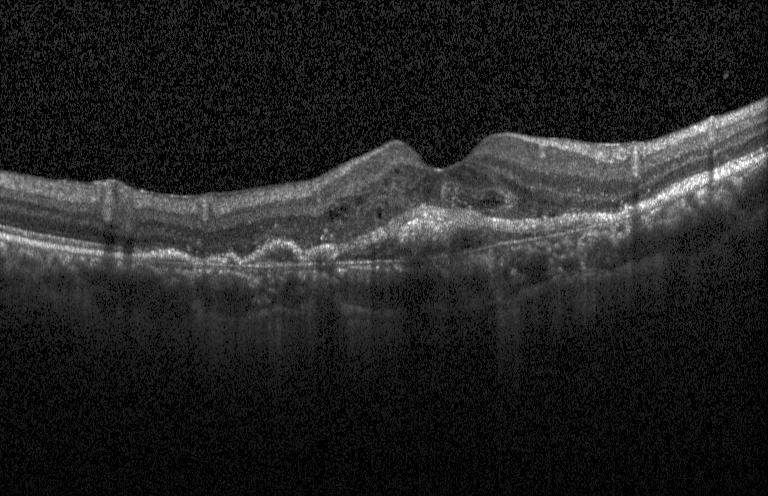 Retinal OCT cross-section. OCT finding: a choroidal neovascular membrane.